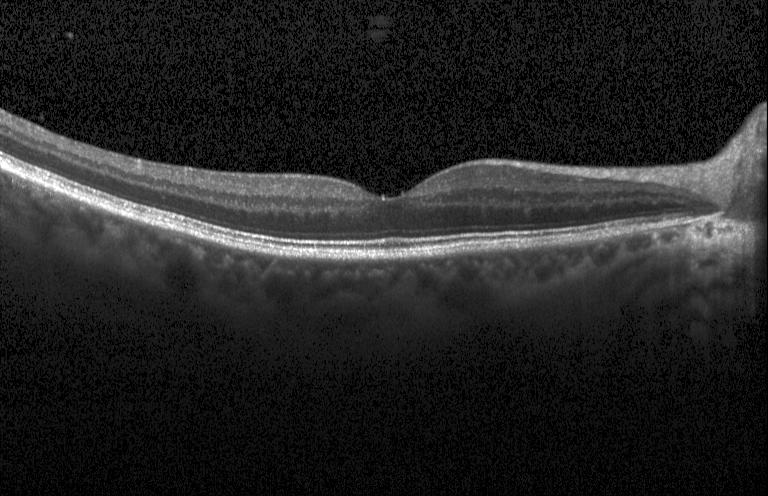

Optical coherence tomography B-scan — Dx: neither choroidal neovascularization, diabetic macular edema, nor drusen.